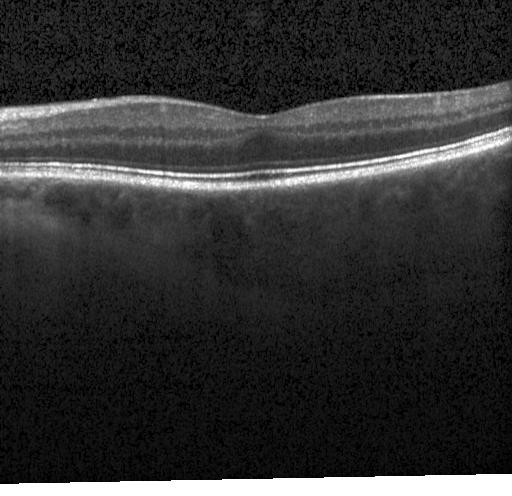

Acquired on a Heidelberg Spectralis · spectral-domain OCT · OCT line scan · through the macula — Impression: no choroidal neovascularization, no diabetic macular edema, and no drusen.